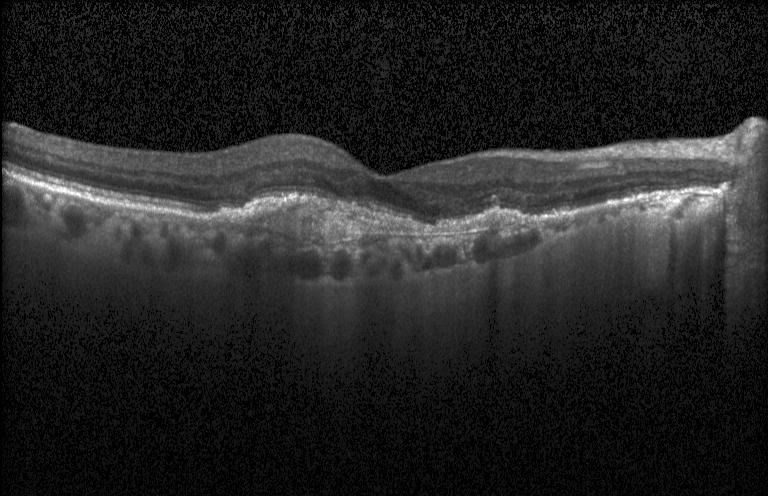
SD-OCT · through the macula · retinal OCT cross-section · Heidelberg Spectralis.
Impression: choroidal neovascularization (CNV).